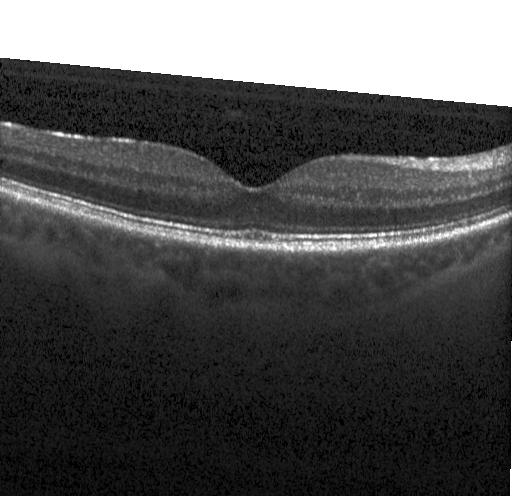
Finding: neither choroidal neovascularization, diabetic macular edema, nor drusen.